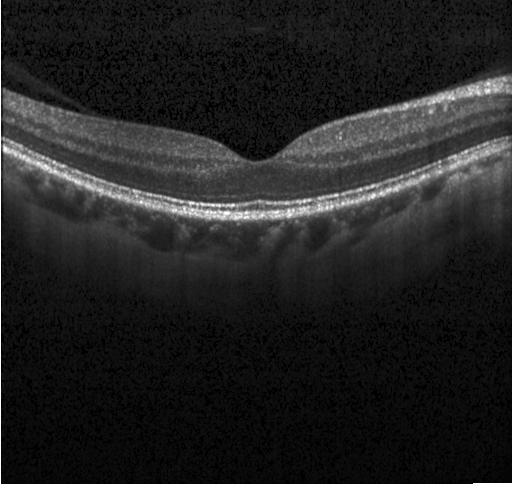

OCT finding: neither CNV, DME, nor drusen.